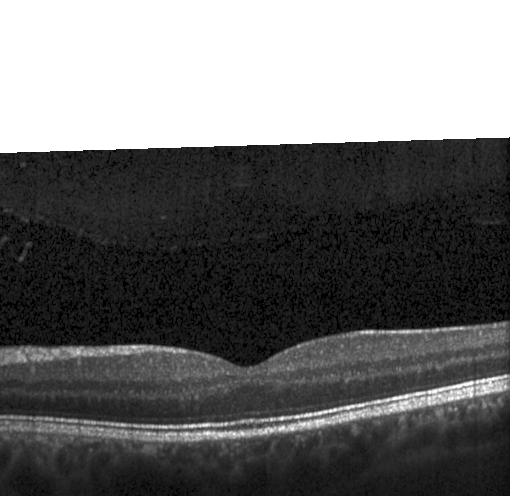 Assessment: neither choroidal neovascularization, diabetic macular edema, nor drusen.